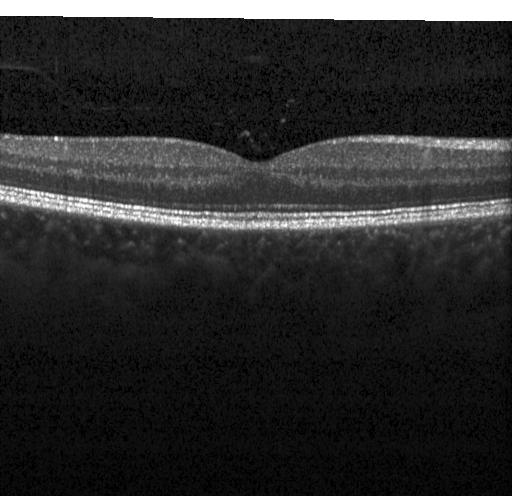 OCT scan showing no choroidal neovascularization, no diabetic macular edema, and no drusen.